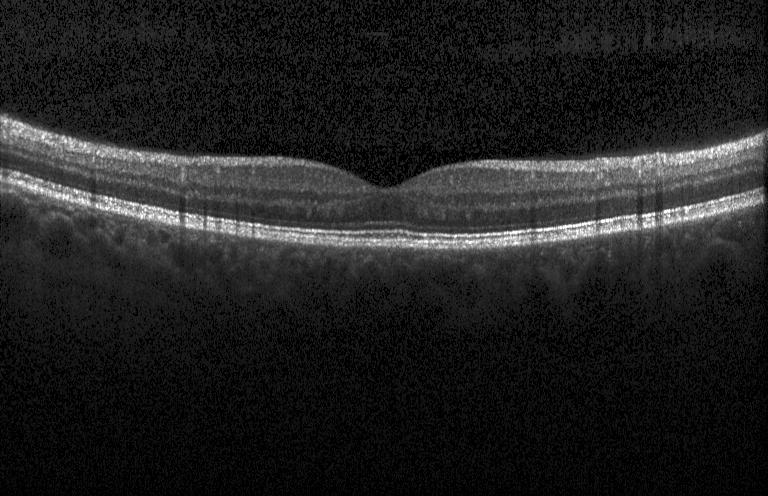 Acquired on a Heidelberg Spectralis · spectral-domain optical coherence tomography · through the macula · OCT B-scan. No CNV, DME, or drusen.